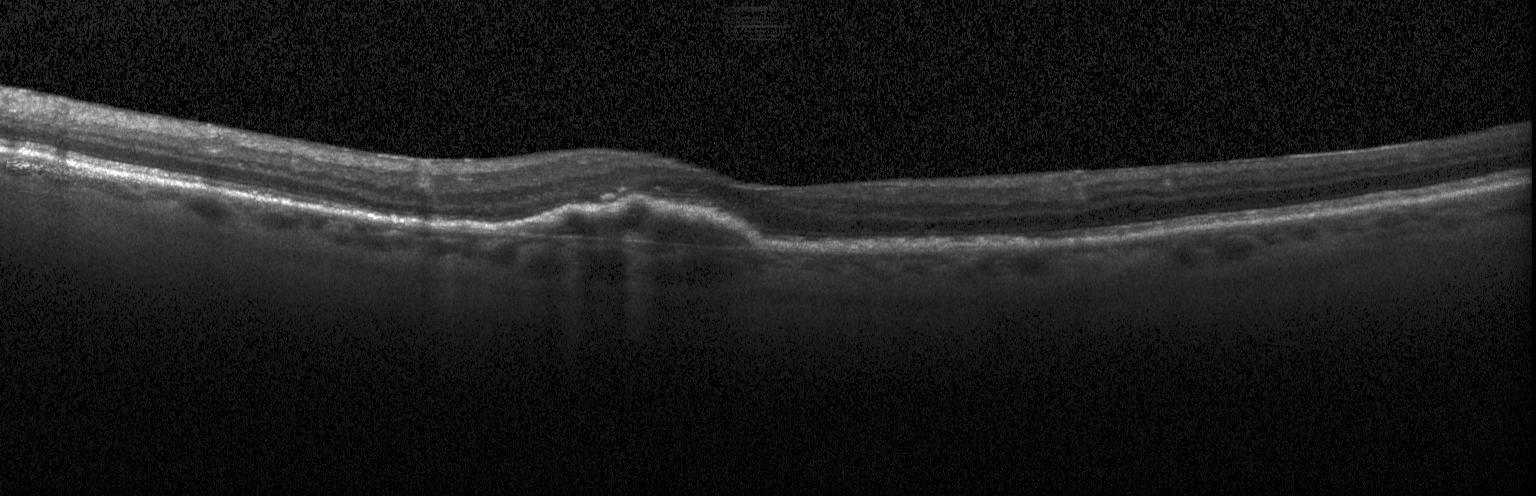

Retinal OCT cross-section. Impression: choroidal neovascularization (CNV).